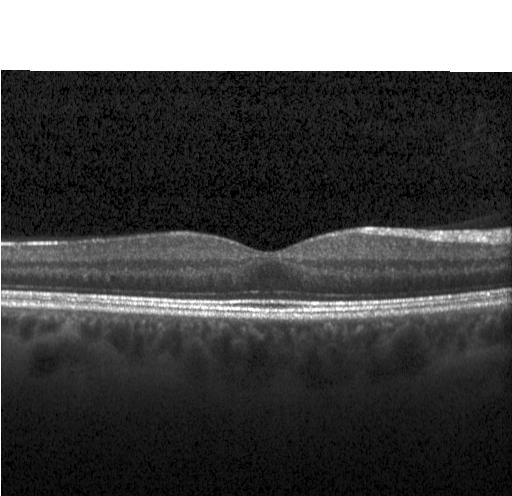

Optical coherence tomography B-scan — Finding: no evidence of choroidal neovascularization, diabetic macular edema, or drusen.